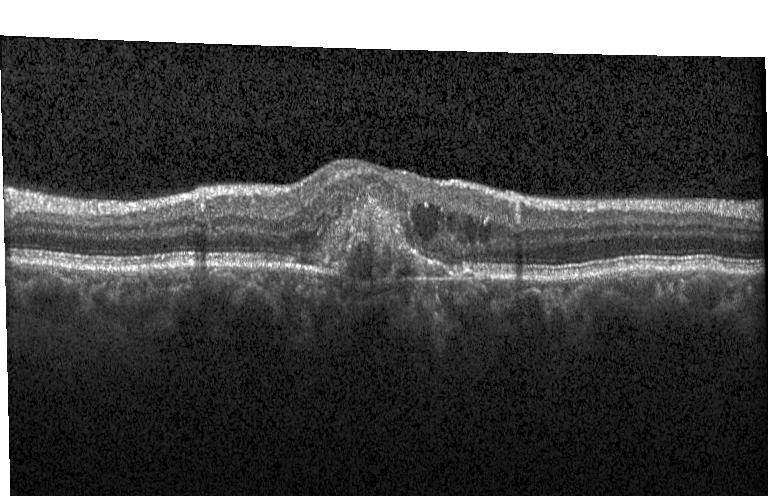

Retinal OCT cross-section; fovea-centered.
This B-scan demonstrates a choroidal neovascular membrane.